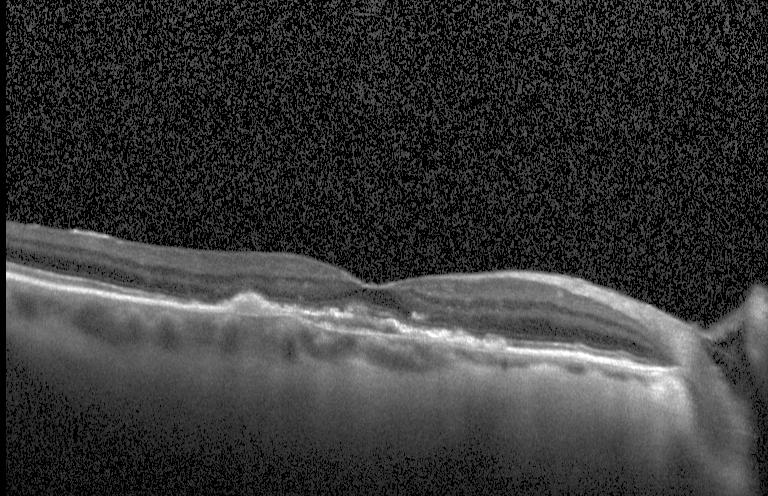
OCT scan showing a choroidal neovascular membrane.